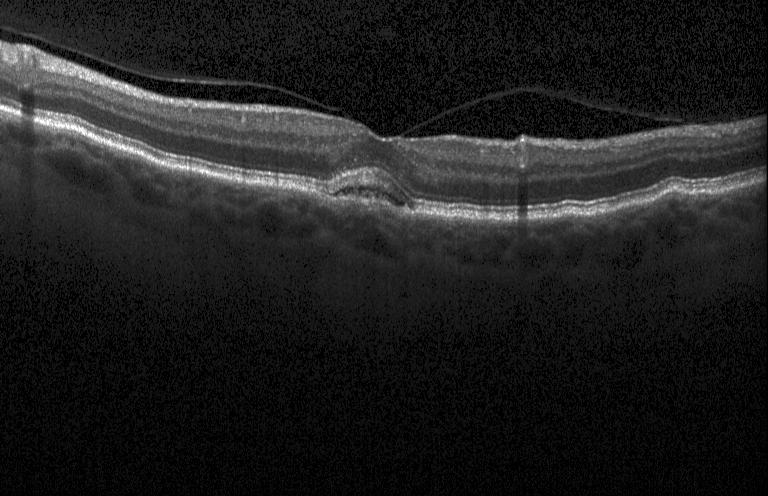

Optical coherence tomography B-scan, spectral-domain OCT
Impression: choroidal neovascularization (CNV).